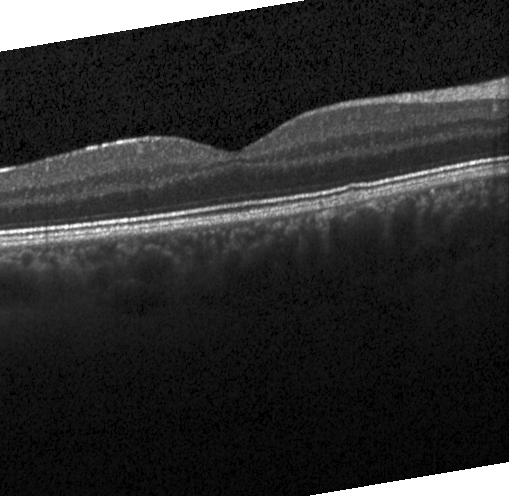 OCT line scan; spectral-domain OCT; Heidelberg Spectralis; centered on the fovea. No choroidal neovascularization, no diabetic macular edema, and no drusen.